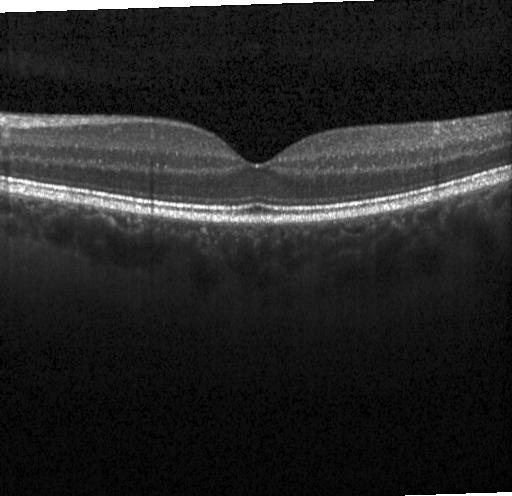 Heidelberg Spectralis. Retinal OCT B-scan. Fovea-centered
The scan shows neither choroidal neovascularization, diabetic macular edema, nor drusen.